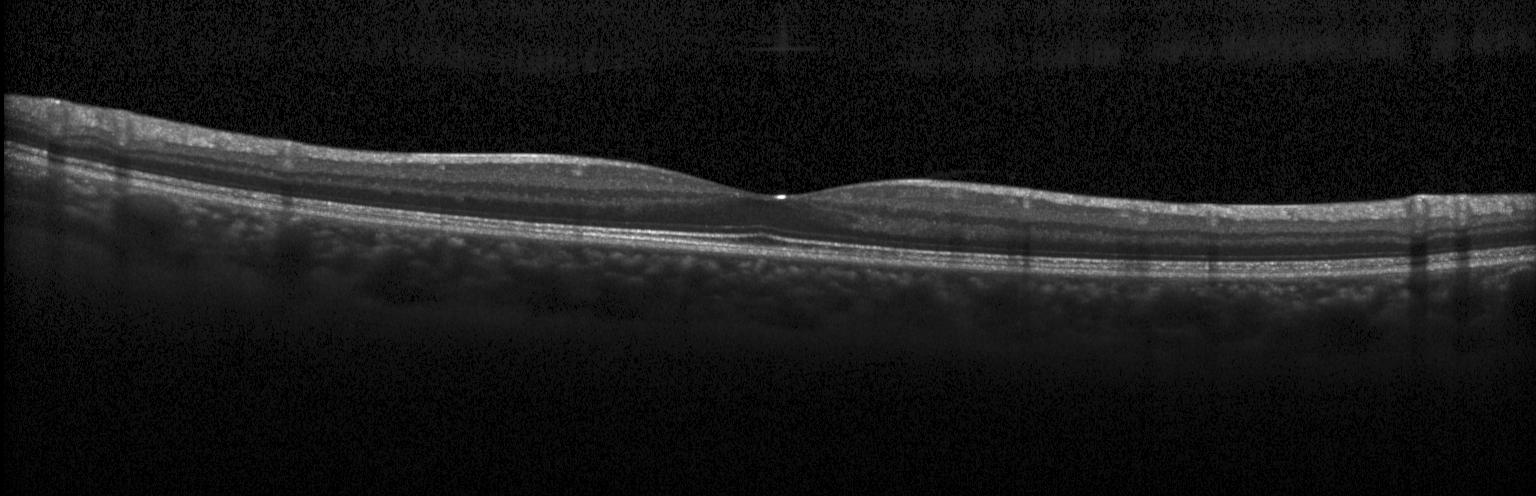
Fovea-centered. OCT line scan. Spectral-domain OCT
Assessment: no evidence of choroidal neovascularization, diabetic macular edema, or drusen.